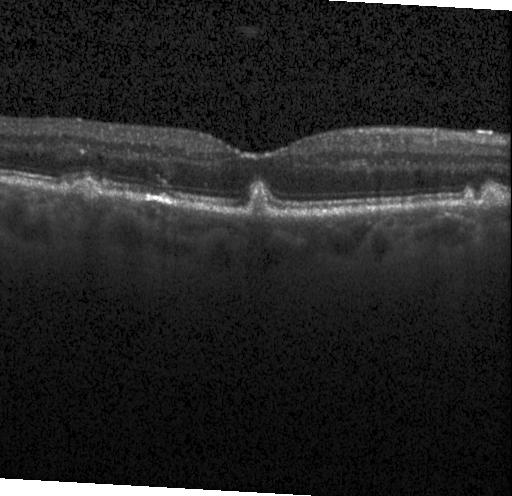 Through the macula, optical coherence tomography scan, spectral-domain optical coherence tomography, Heidelberg Spectralis.
Finding: sub-RPE drusenoid deposits.